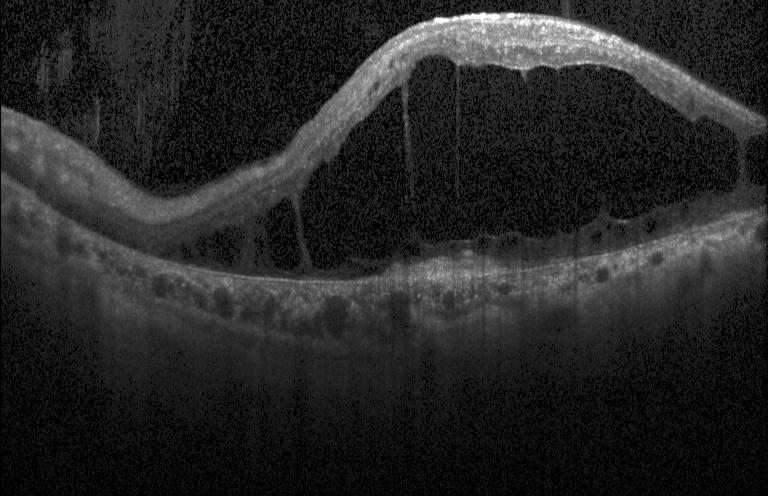
Retinal OCT B-scan. Spectral-domain optical coherence tomography. Heidelberg Spectralis OCT system
Macular OCT: diabetic macular edema.